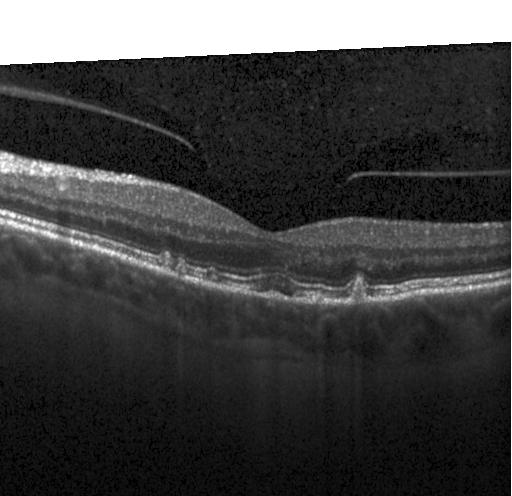

Centered on the fovea. Optical coherence tomography B-scan
Finding: drusen.